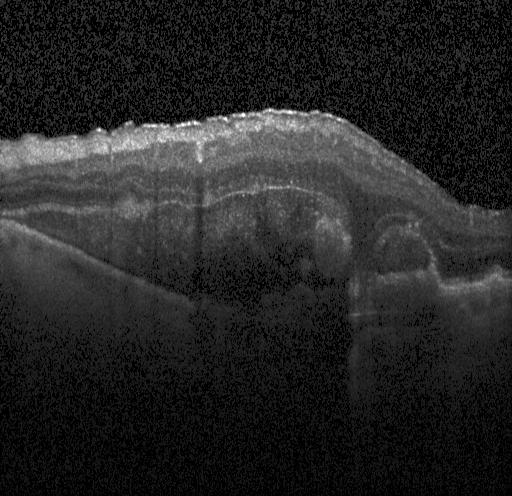
Macular scan, optical coherence tomography scan.
Finding: choroidal neovascularization.